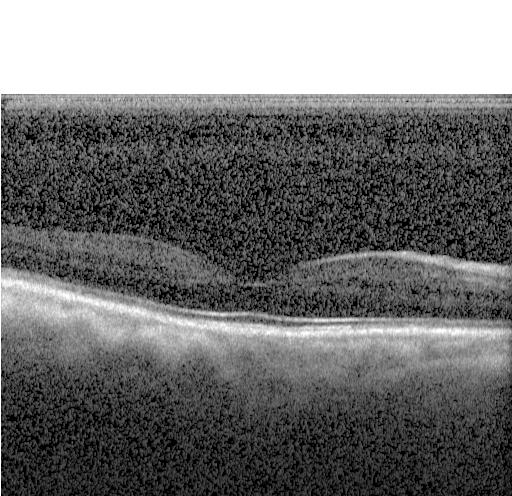

OCT B-scan; Heidelberg Spectralis OCT system; through the macula; spectral-domain OCT. The scan shows no evidence of CNV, DME, or drusen.